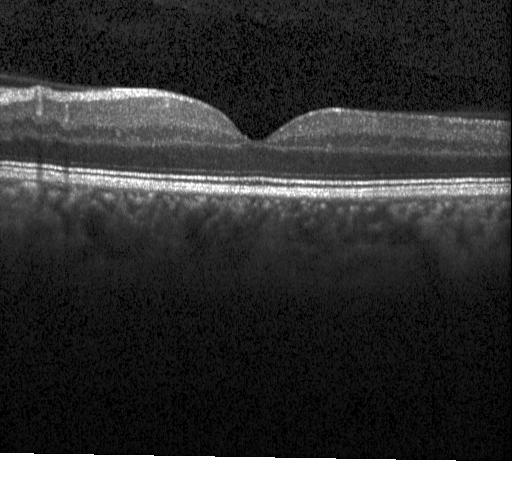 Optical coherence tomography B-scan, Heidelberg Spectralis OCT system. Diagnosis: no CNV, no DME, and no drusen.